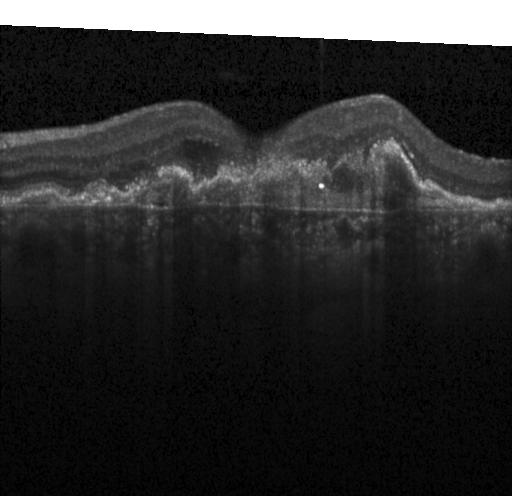
Finding: a choroidal neovascular membrane.